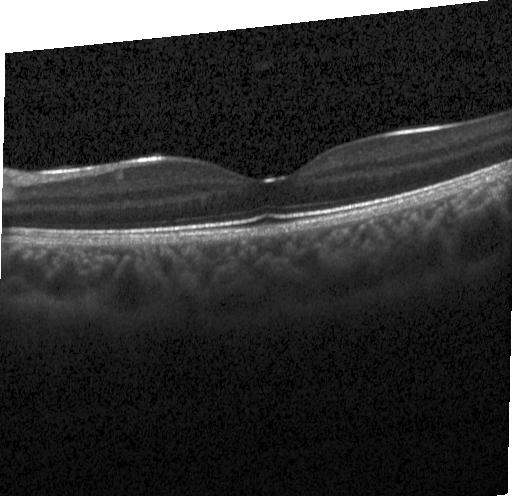

Impression: neither choroidal neovascularization, diabetic macular edema, nor drusen.